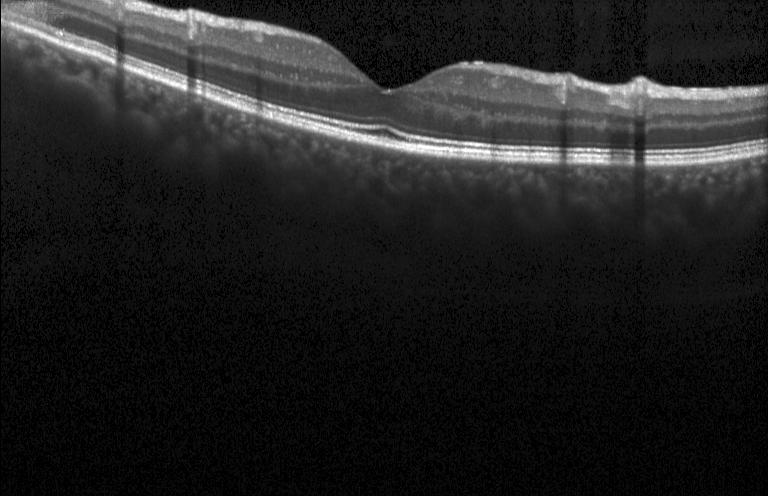
Impression: neither CNV, DME, nor drusen.